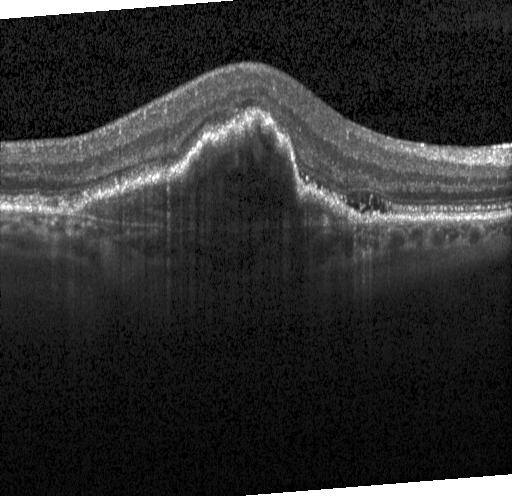 Impression: a choroidal neovascular membrane.